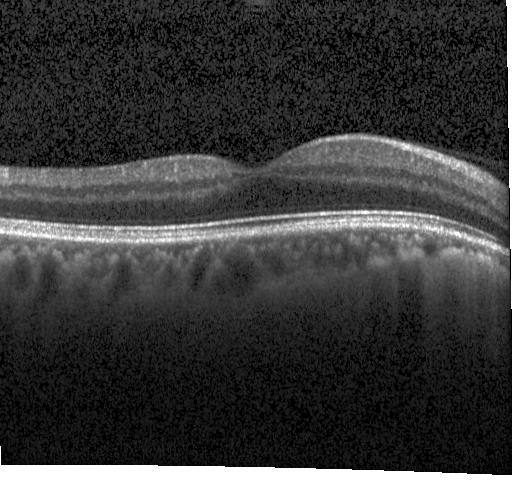
Diagnosis: no choroidal neovascularization, diabetic macular edema, or drusen.